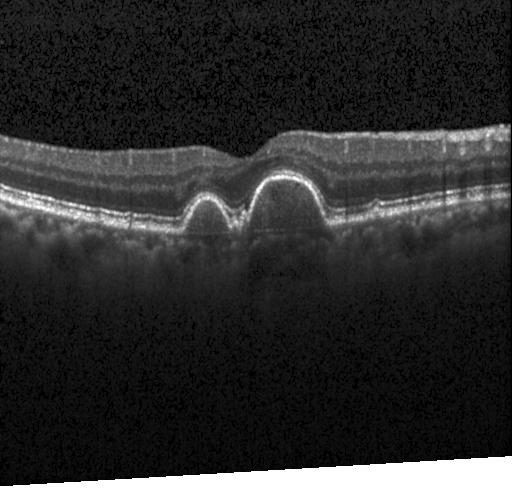 Optical coherence tomography B-scan — Diagnosis: drusen.